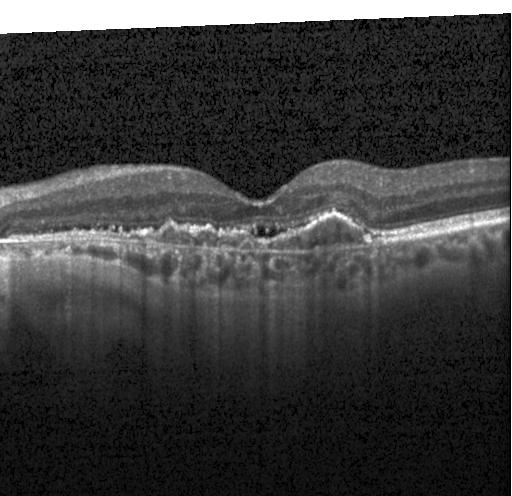

This B-scan demonstrates a choroidal neovascular membrane.